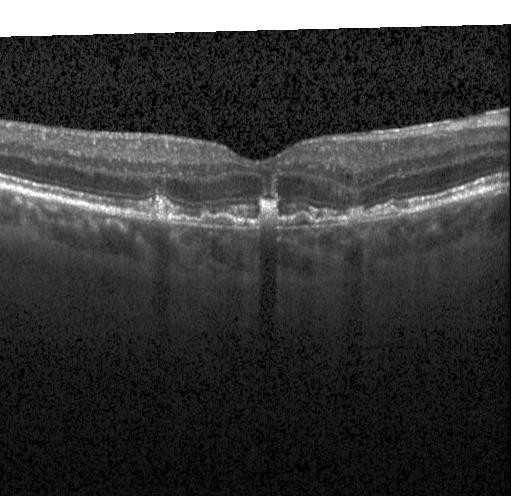
Dx: CNV.